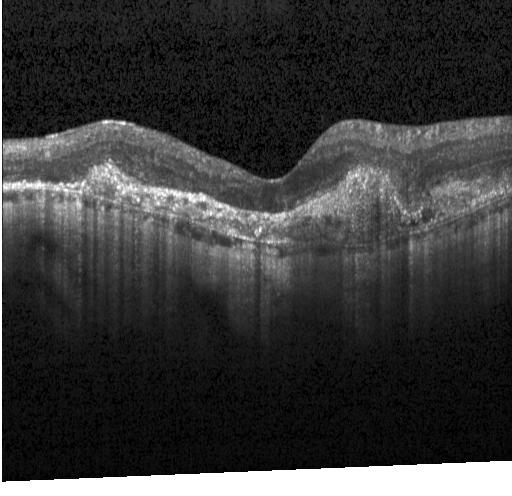

Retinal OCT cross-section showing choroidal neovascularization.